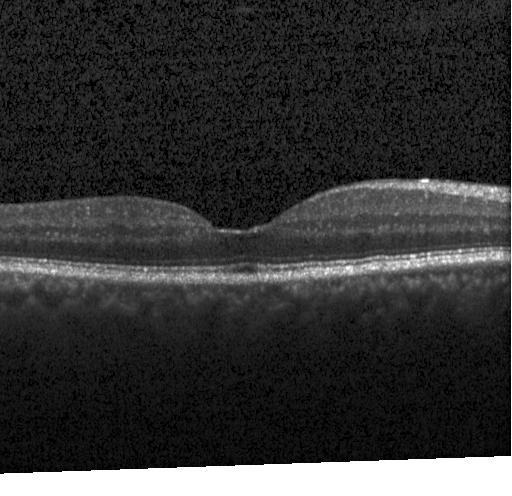

Heidelberg Spectralis. OCT B-scan. Spectral-domain OCT. Centered on the fovea.
Impression: no evidence of CNV, DME, or drusen.